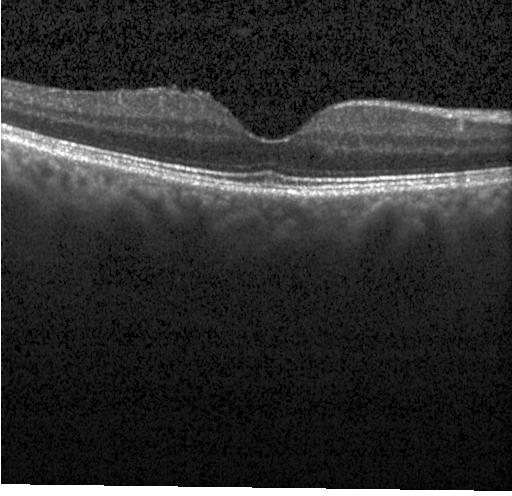
Macular OCT: no choroidal neovascularization, no diabetic macular edema, and no drusen.